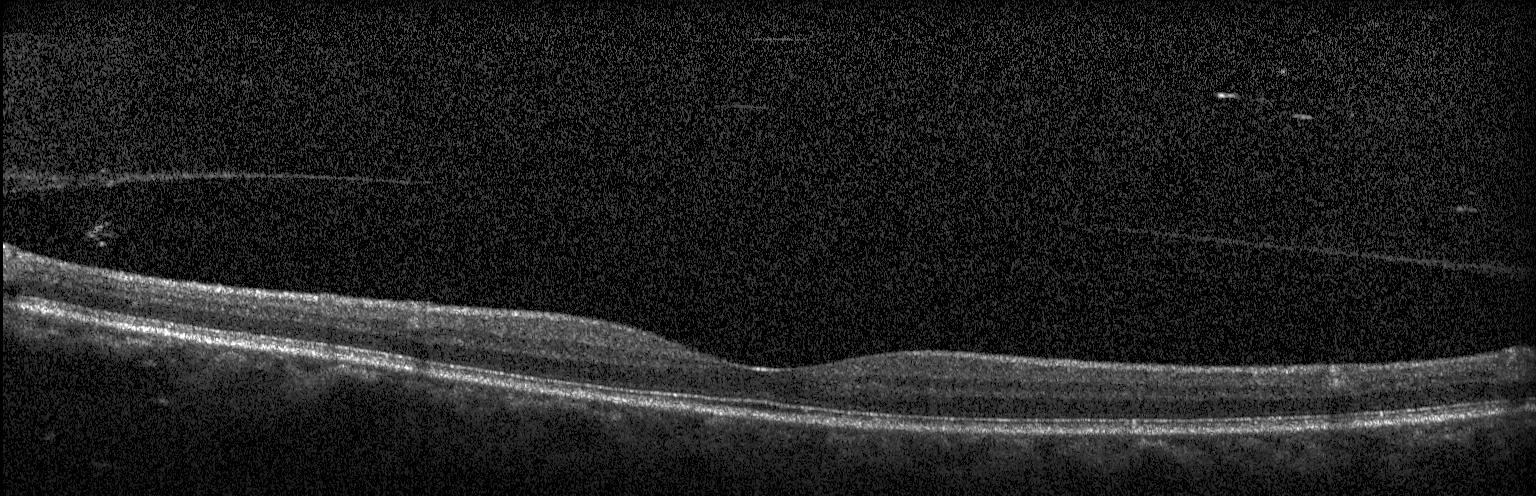

Retinal OCT cross-section showing no choroidal neovascularization, diabetic macular edema, or drusen.